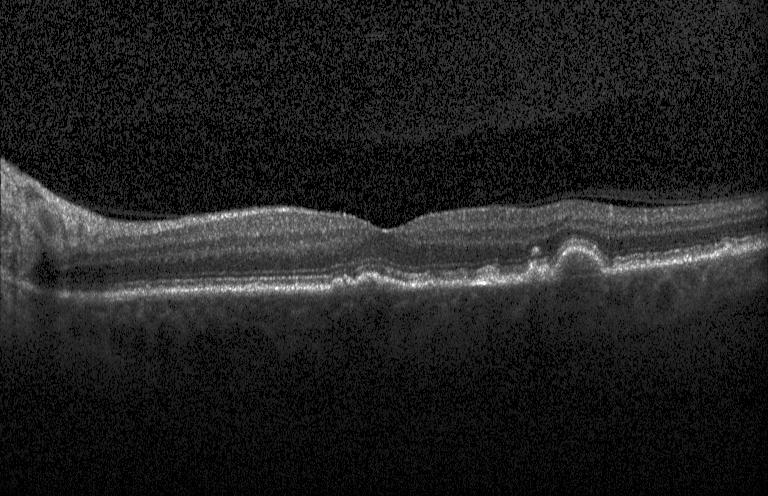

Horizontal scan through the fovea. Spectral-domain OCT. Heidelberg Spectralis OCT system. Retinal OCT cross-section
Impression: multiple drusen.